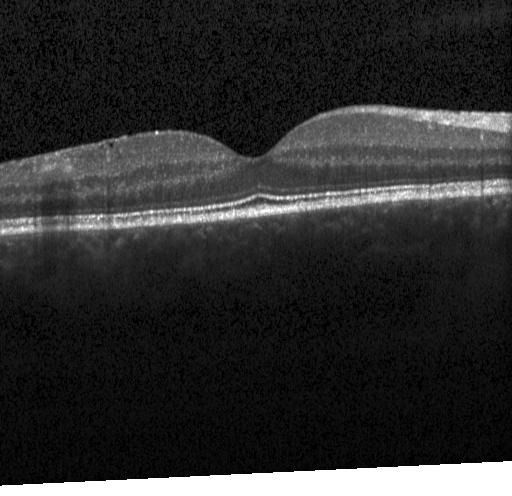

Retinal OCT B-scan. Spectral-domain OCT. Macular scan — Finding: neither choroidal neovascularization, diabetic macular edema, nor drusen.